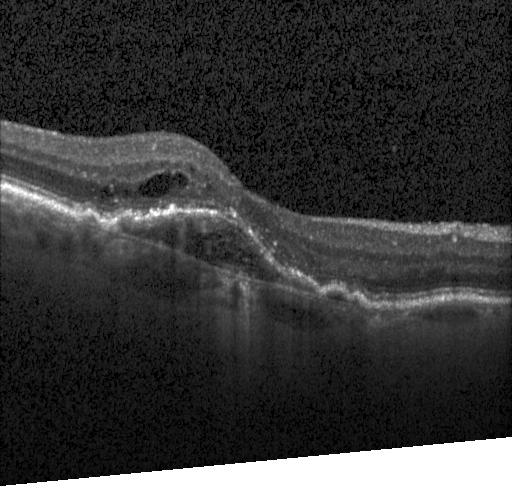

Assessment: choroidal neovascularization (CNV).